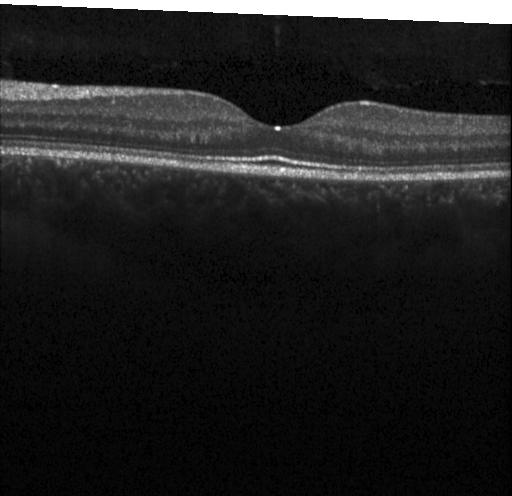 Retinal OCT cross-section. Diagnosis: no evidence of CNV, DME, or drusen.